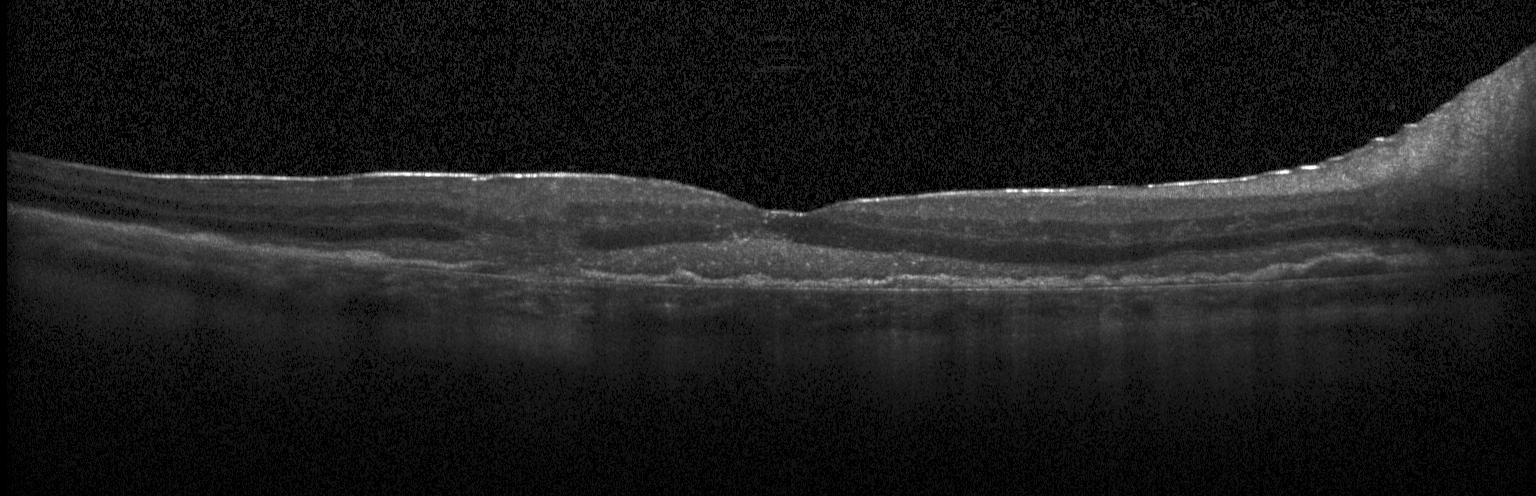

OCT scan showing a choroidal neovascular membrane.